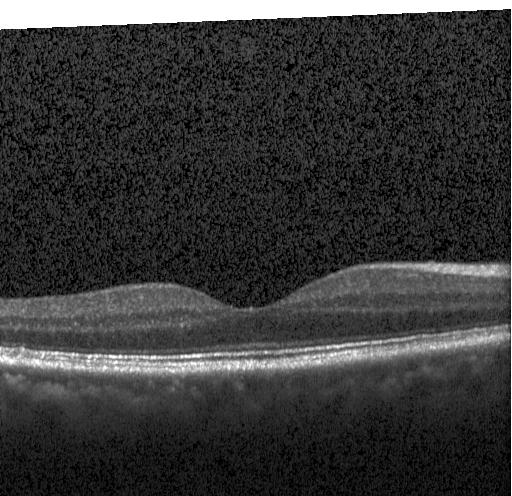 OCT B-scan — Impression: neither choroidal neovascularization, diabetic macular edema, nor drusen.